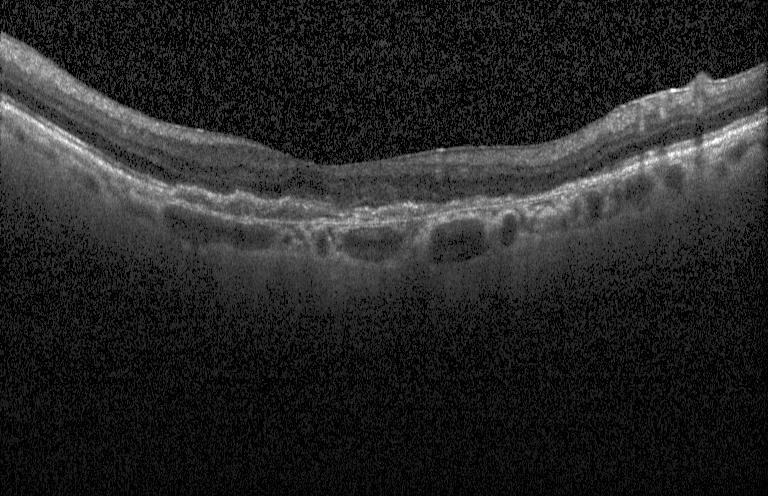

Acquired on a Heidelberg Spectralis · OCT line scan.
Impression: a choroidal neovascular membrane.